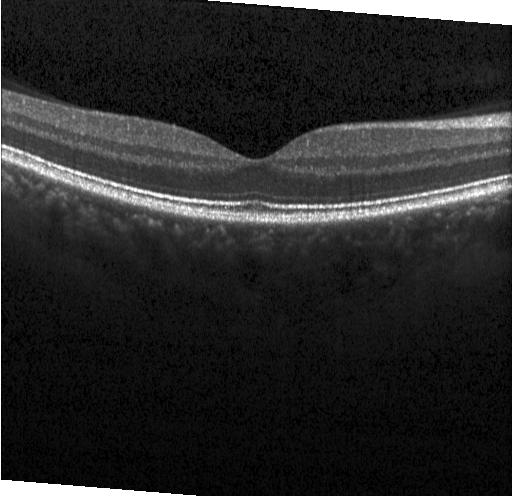
The scan shows neither choroidal neovascularization, diabetic macular edema, nor drusen.